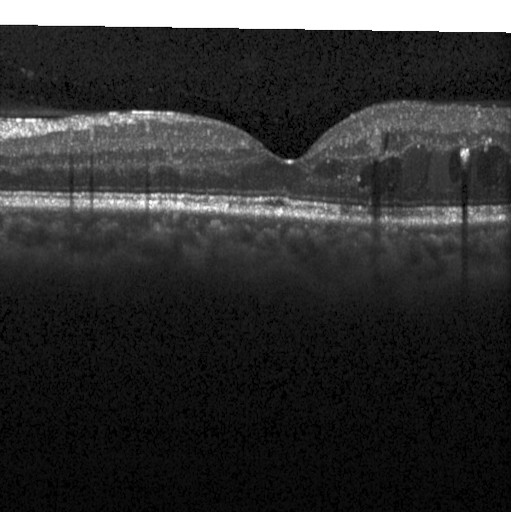 Instrument: Heidelberg Spectralis, macular scan, retinal OCT B-scan — Diagnosis: DME.